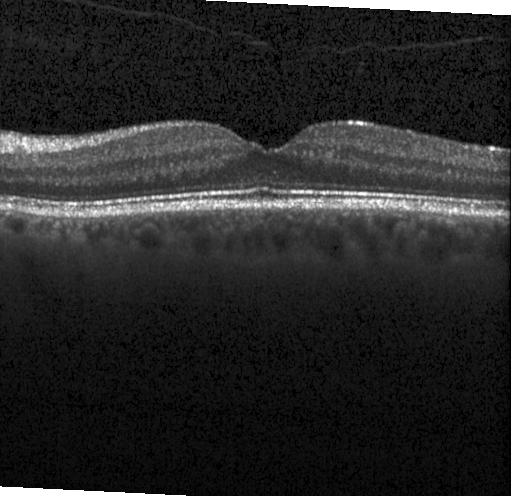
Retinal OCT cross-section showing neither choroidal neovascularization, diabetic macular edema, nor drusen.